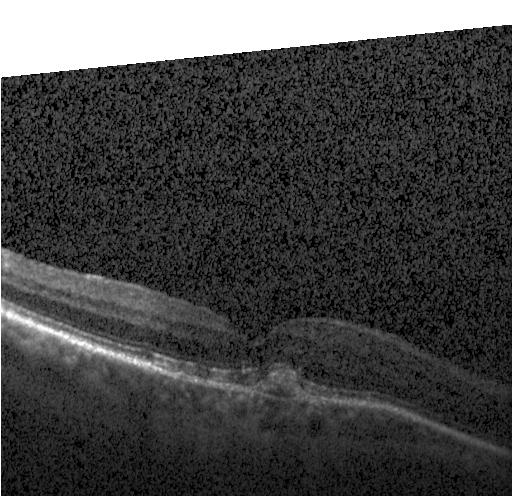 Horizontal scan through the fovea; optical coherence tomography scan — Finding: a choroidal neovascular membrane.